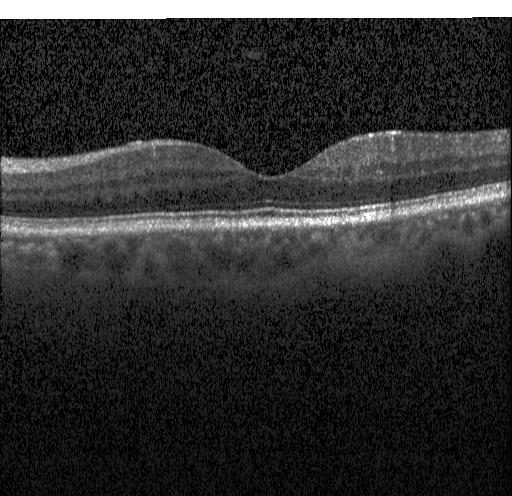
Macular scan. Optical coherence tomography scan. SD-OCT. Acquired on a Heidelberg Spectralis. Impression: neither choroidal neovascularization, diabetic macular edema, nor drusen.